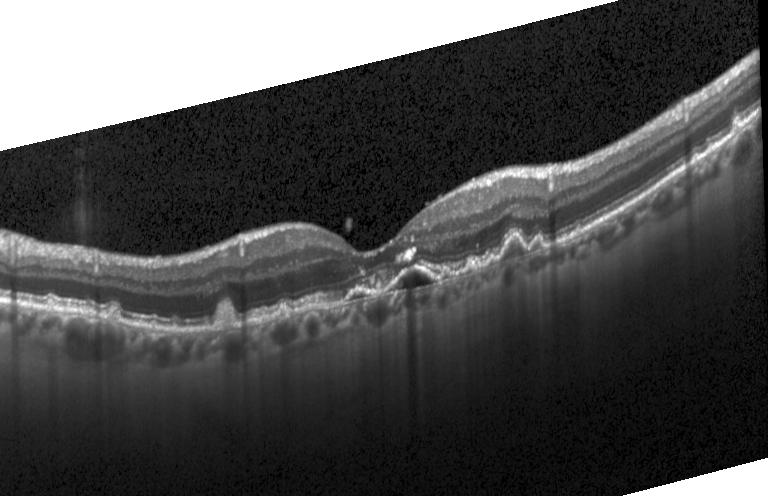

Finding: choroidal neovascularization (CNV).